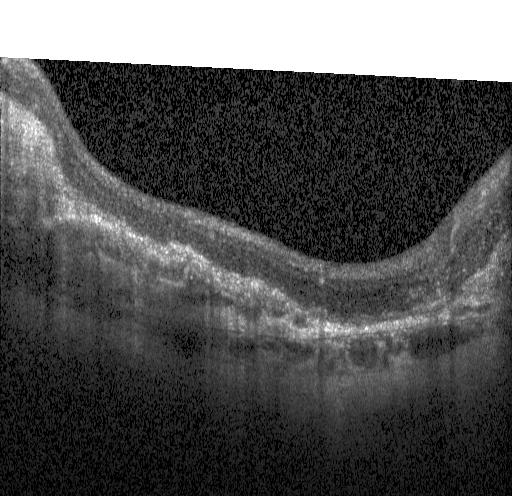

SD-OCT, through the macula, optical coherence tomography scan, acquired on a Heidelberg Spectralis.
Dx: choroidal neovascularization (CNV).